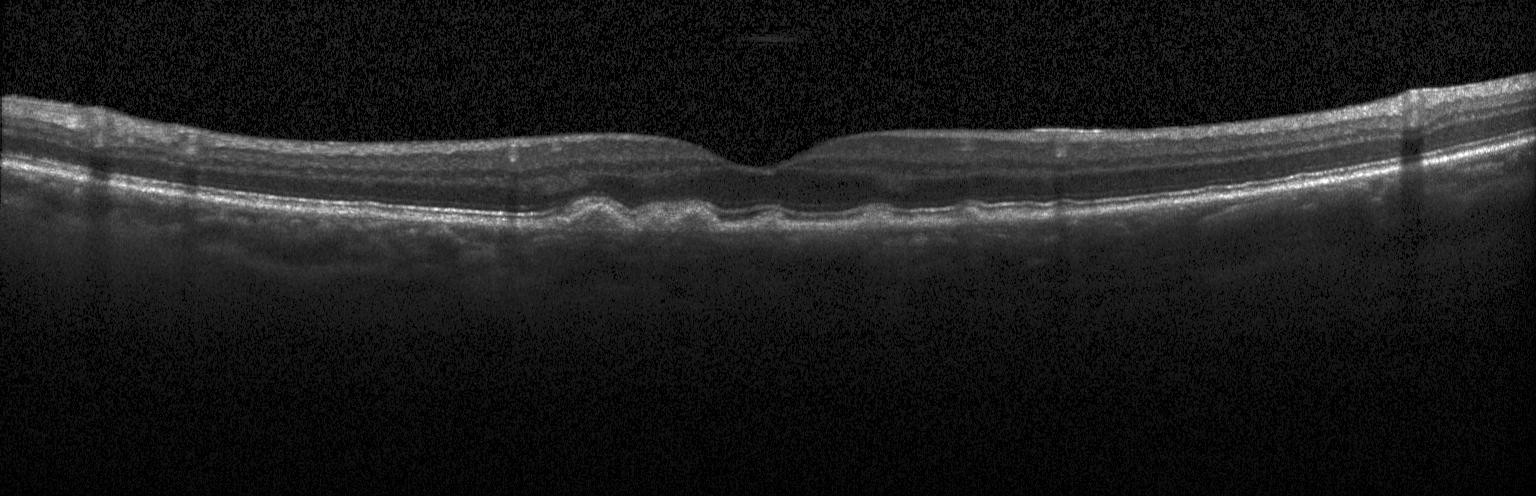
Retinal OCT B-scan — Finding: drusen.